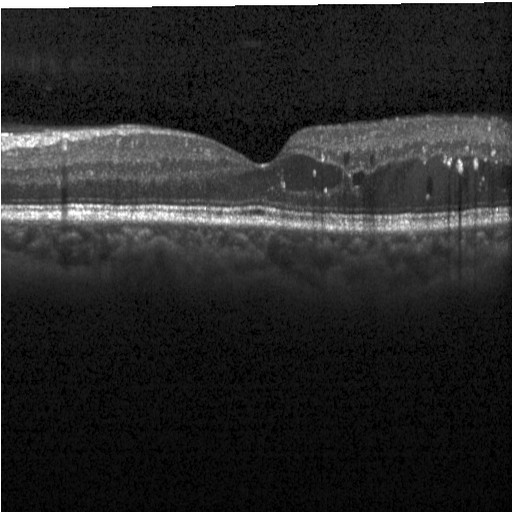 Instrument: Heidelberg Spectralis. Through the macula. OCT B-scan — Finding: diabetic macular edema (DME).